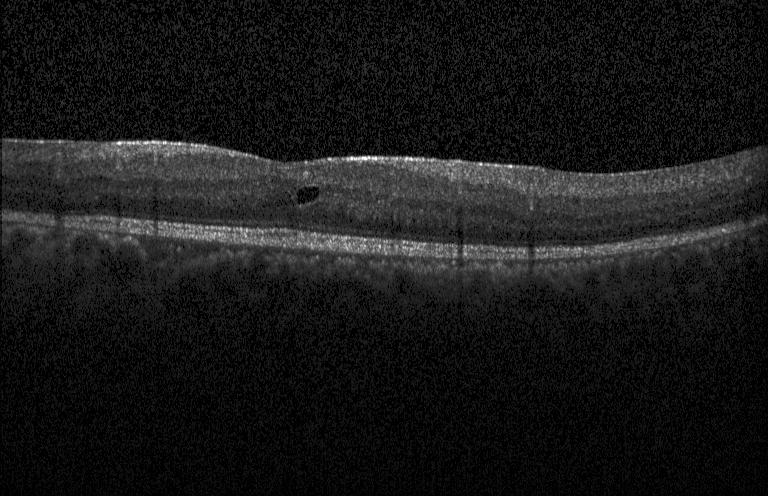
OCT line scan, horizontal scan through the fovea.
This B-scan demonstrates DME.